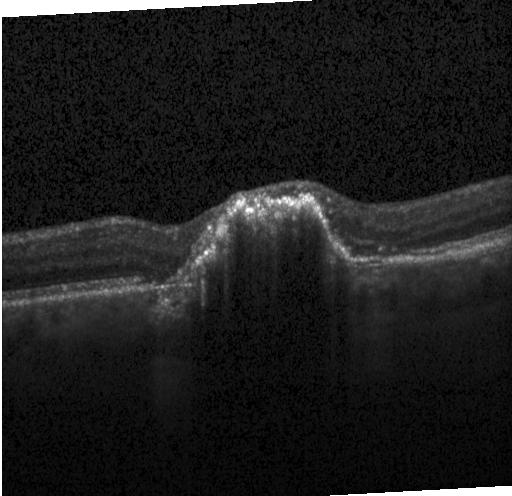

Diagnosis: choroidal neovascularization (CNV).